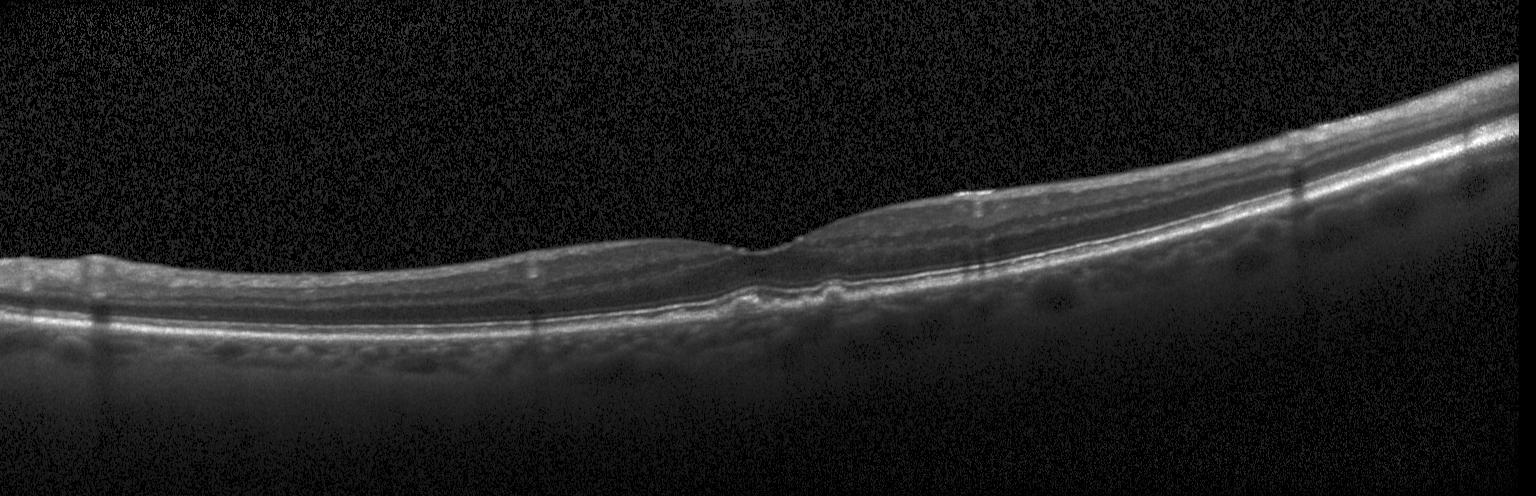
Dx: multiple drusen.